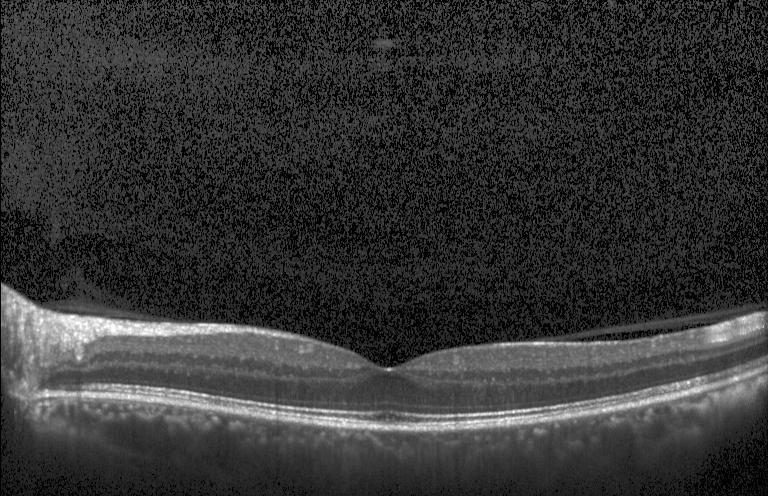
Impression: no choroidal neovascularization, no diabetic macular edema, and no drusen.